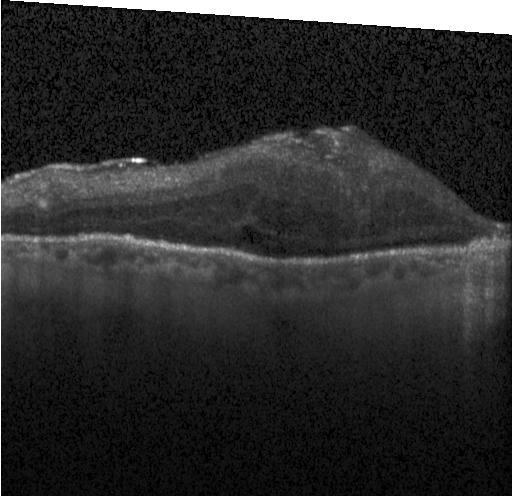 Macular OCT demonstrating a choroidal neovascular membrane.